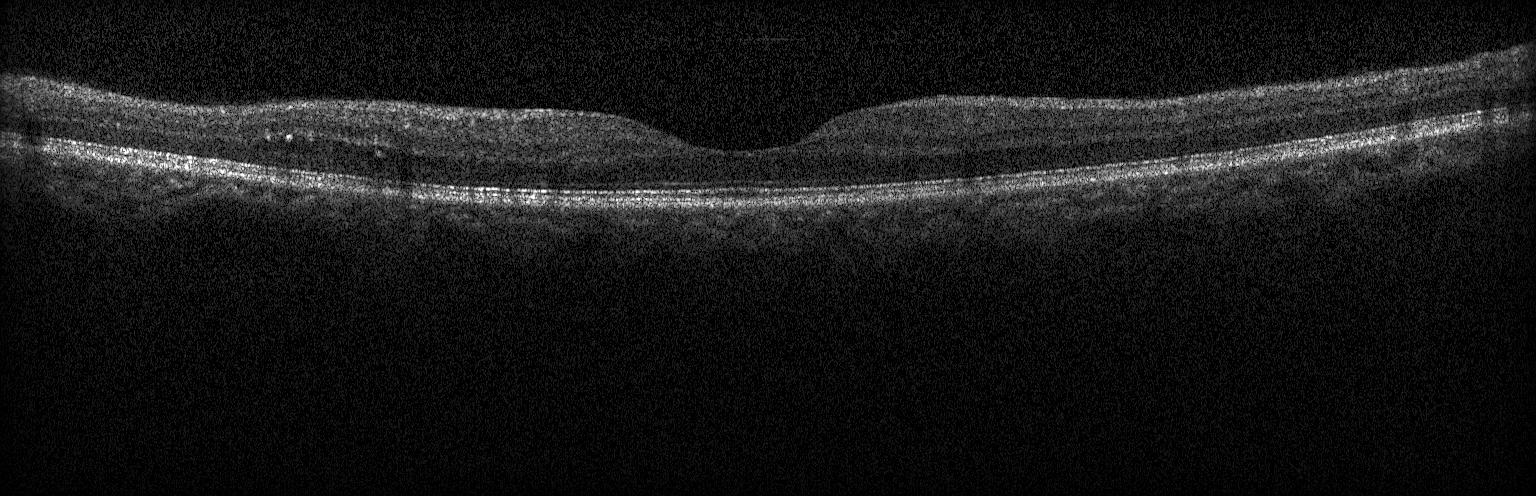 Acquired on a Heidelberg Spectralis. Optical coherence tomography B-scan. Finding: no evidence of choroidal neovascularization, diabetic macular edema, or drusen.